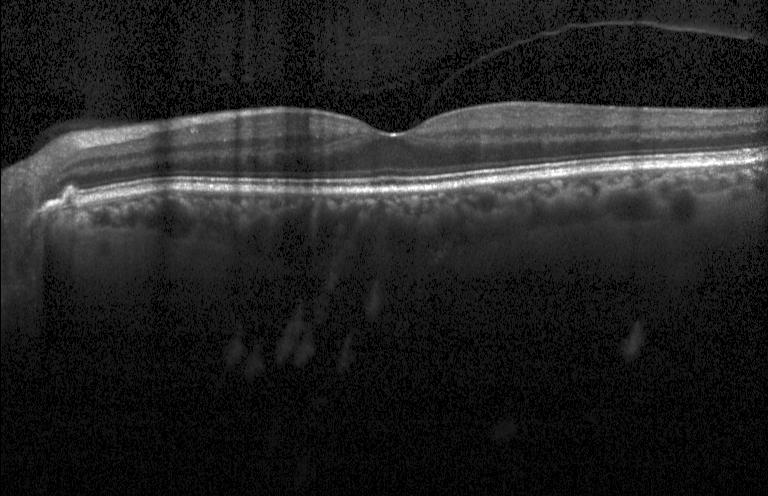
Finding: no choroidal neovascularization, diabetic macular edema, or drusen.